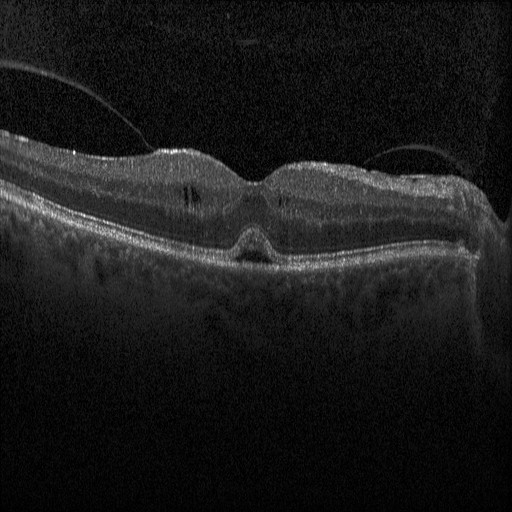

Optical coherence tomography B-scan; spectral-domain OCT — Diagnosis: diabetic macular edema.